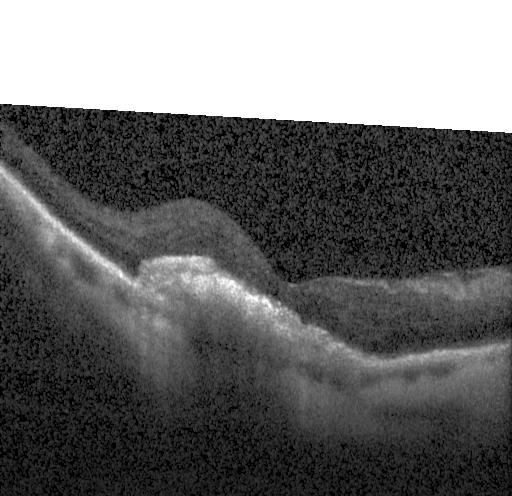 The scan shows CNV.